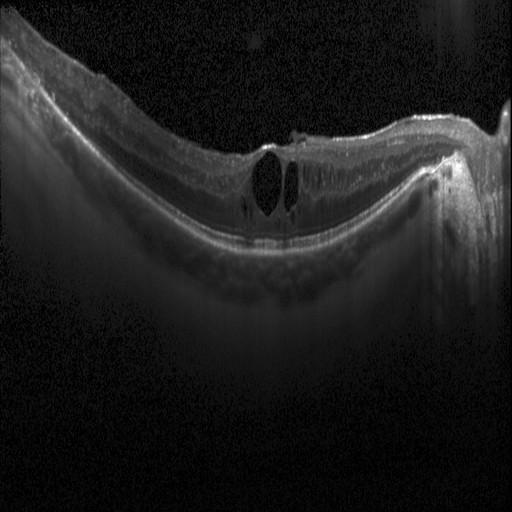 OCT finding: diabetic macular edema.